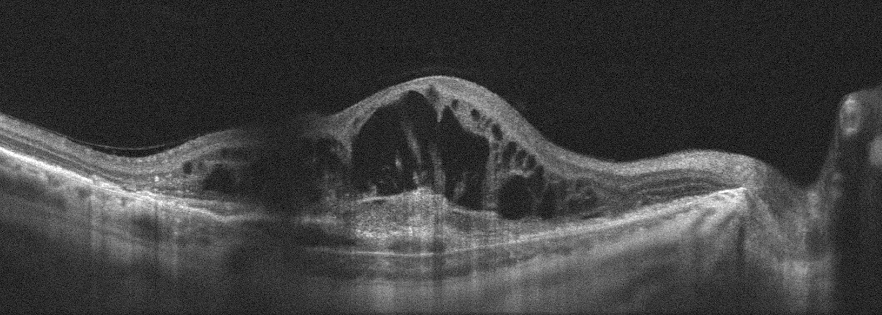

Right eye; optical coherence tomography scan — Age-related macular degeneration (AMD).